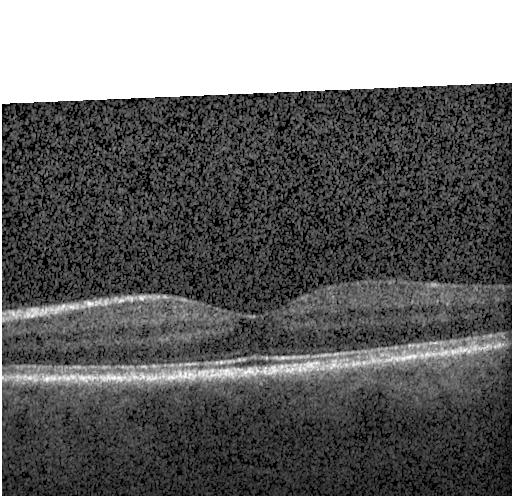
SD-OCT. Optical coherence tomography scan — This B-scan demonstrates no CNV, DME, or drusen.